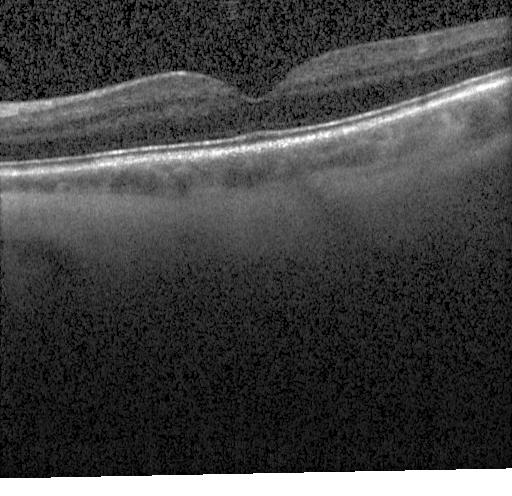

Retinal OCT cross-section · spectral-domain optical coherence tomography · macular scan.
The scan shows neither choroidal neovascularization, diabetic macular edema, nor drusen.